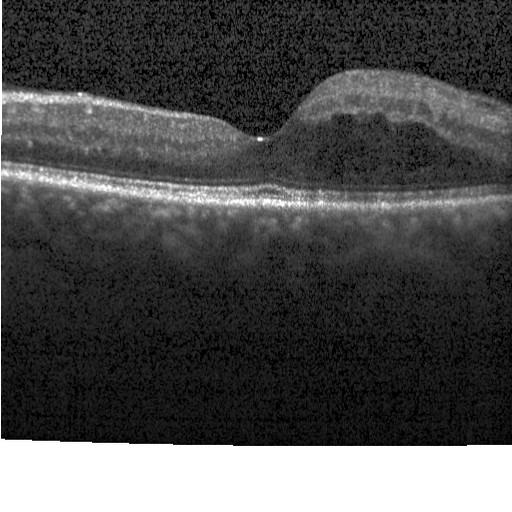
Optical coherence tomography B-scan.
Finding: diabetic macular edema (DME).